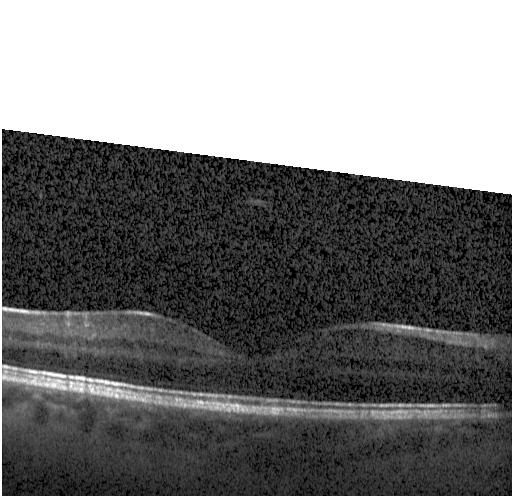

This B-scan demonstrates no choroidal neovascularization, diabetic macular edema, or drusen.